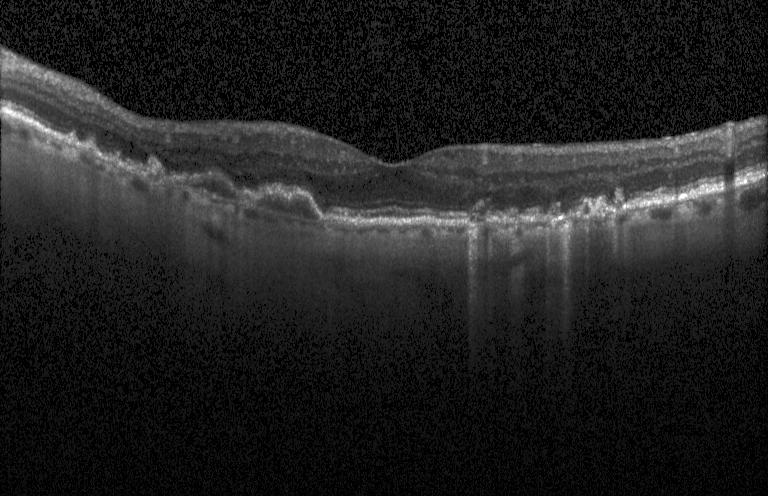 Spectral-domain OCT. OCT line scan. Finding: choroidal neovascularization.